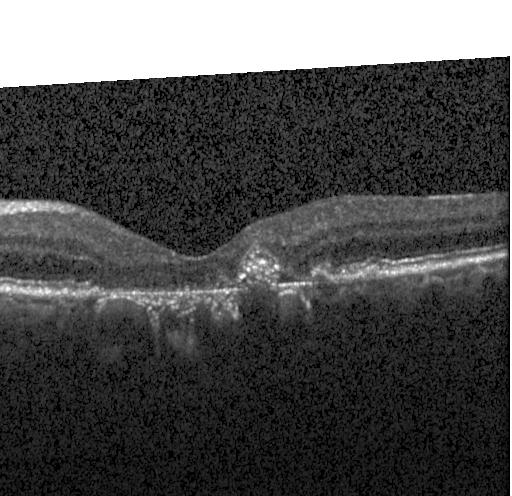

Diagnosis: choroidal neovascularization.